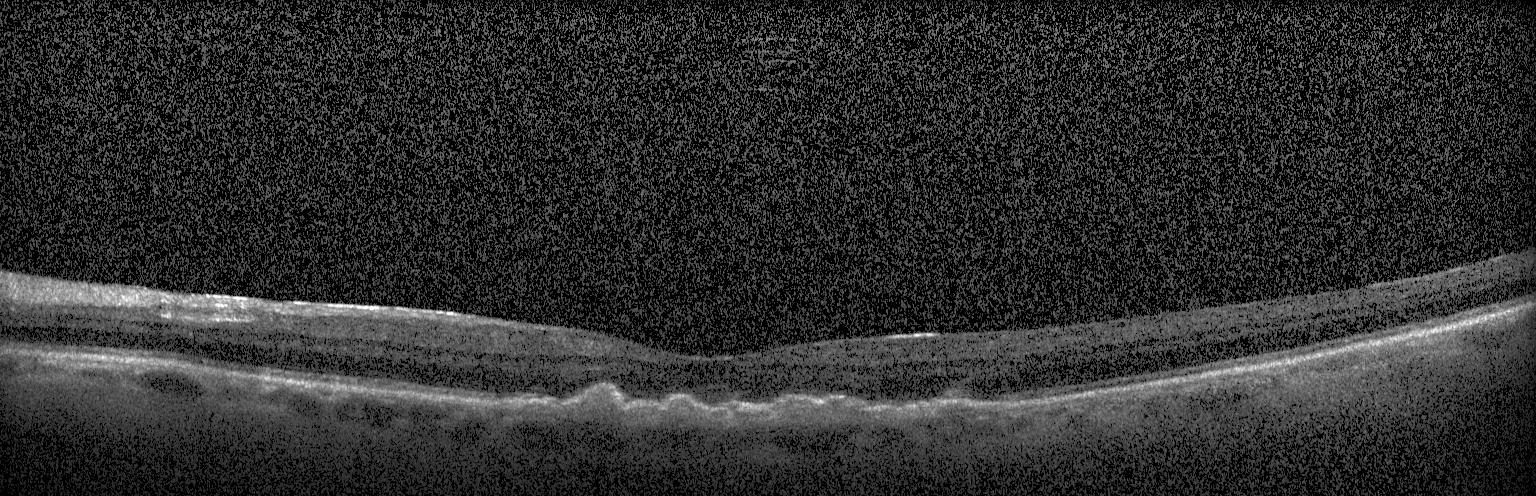

Through the macula, optical coherence tomography B-scan.
Assessment: drusen.